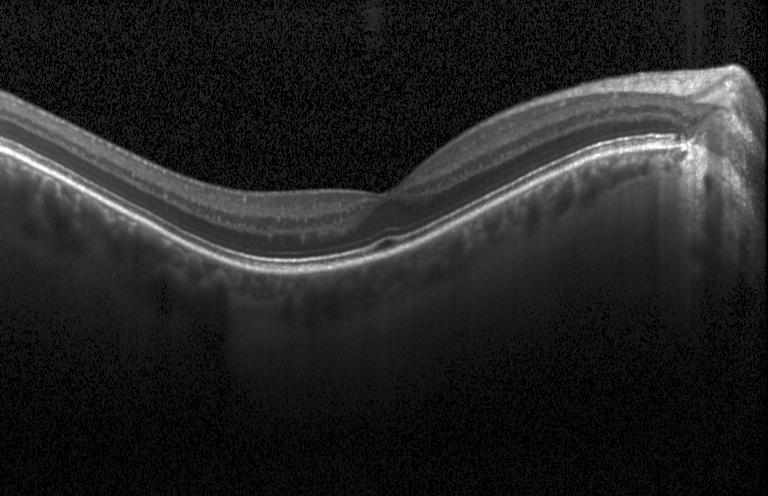 Spectral-domain OCT B-scan: no evidence of choroidal neovascularization, diabetic macular edema, or drusen.